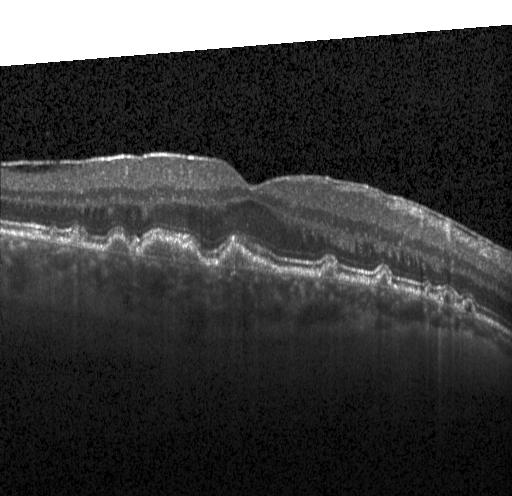 Optical coherence tomography B-scan — Diagnosis: a choroidal neovascular membrane.